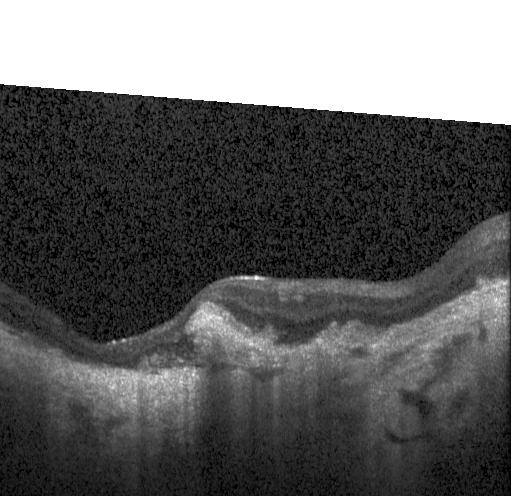
Macular OCT: a choroidal neovascular membrane.